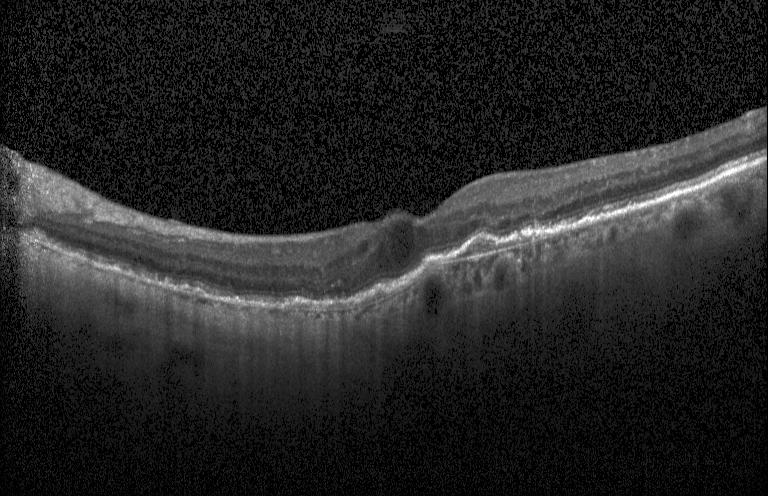
Optical coherence tomography B-scan. Assessment: CNV.